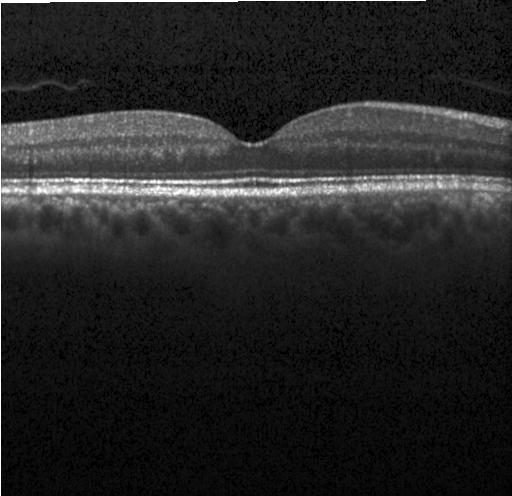

Optical coherence tomography scan; spectral-domain optical coherence tomography
Diagnosis: neither CNV, DME, nor drusen.